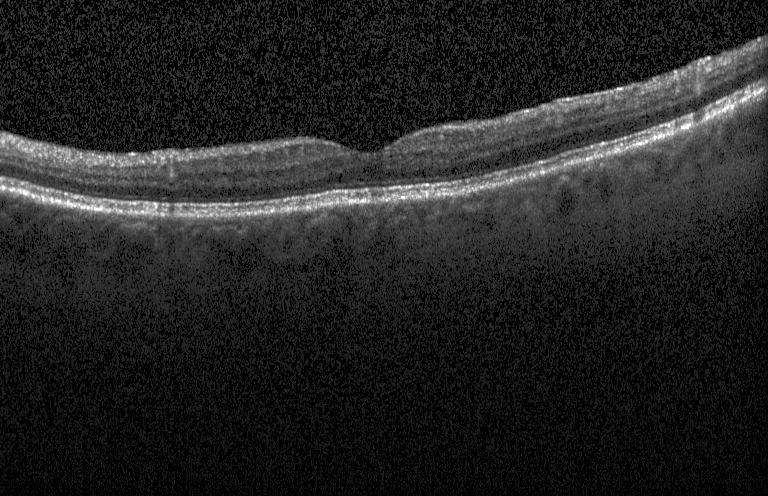

OCT B-scan. The scan shows neither choroidal neovascularization, diabetic macular edema, nor drusen.